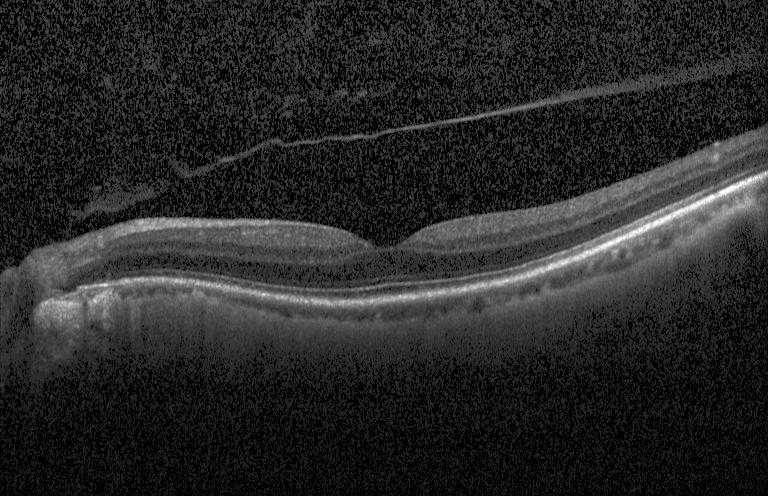 This B-scan demonstrates neither choroidal neovascularization, diabetic macular edema, nor drusen.